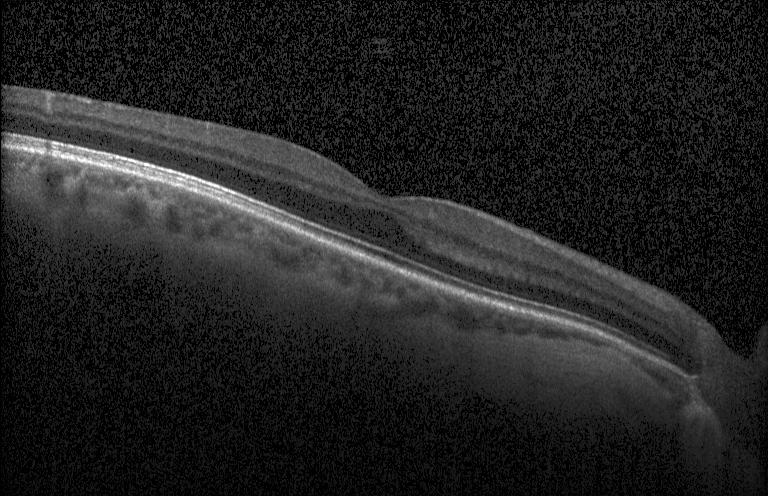 OCT B-scan. OCT finding: neither choroidal neovascularization, diabetic macular edema, nor drusen.